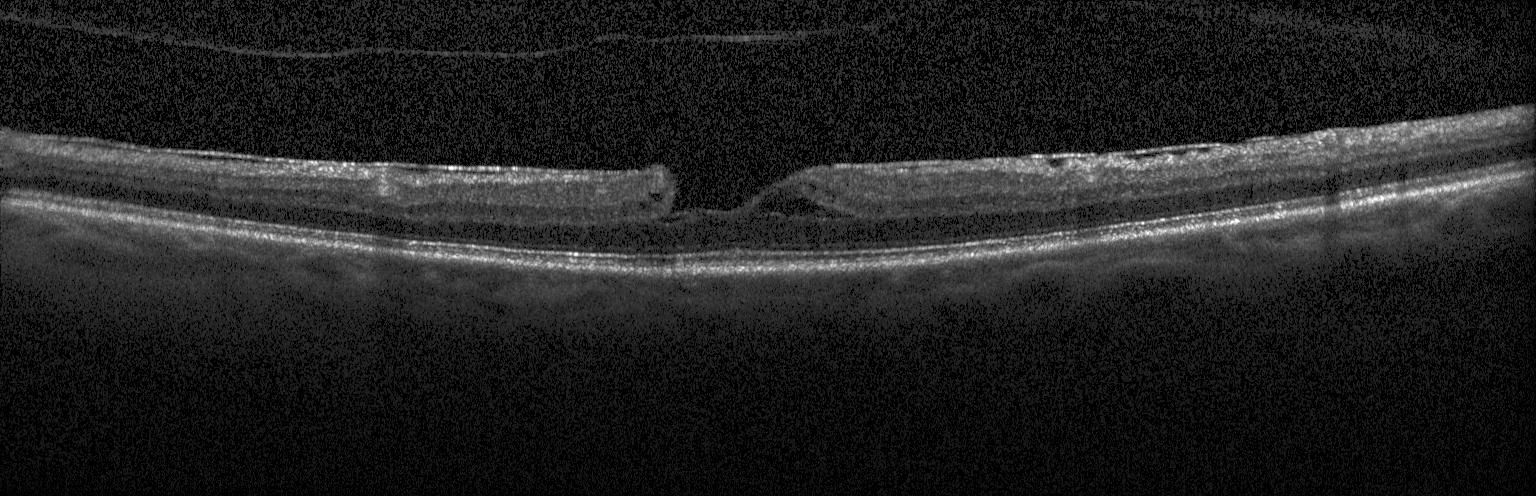 Instrument: Heidelberg Spectralis, spectral-domain optical coherence tomography, macular scan, retinal OCT B-scan.
Finding: diabetic macular edema (DME).